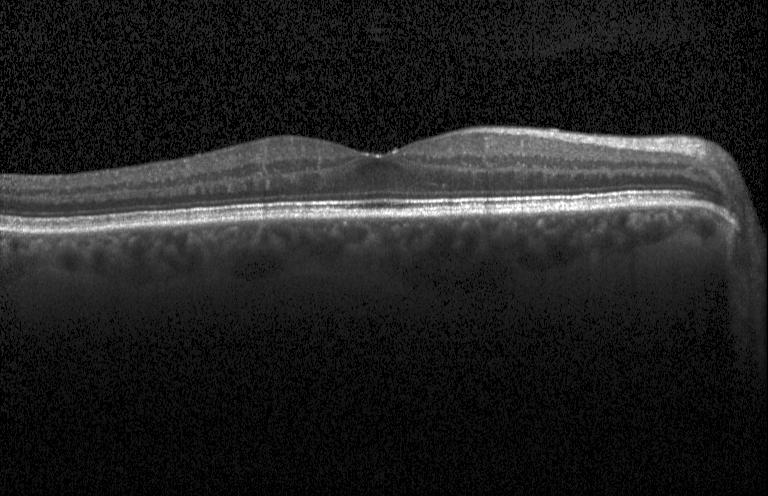
Macular scan; retinal OCT B-scan — This B-scan demonstrates no CNV, no DME, and no drusen.